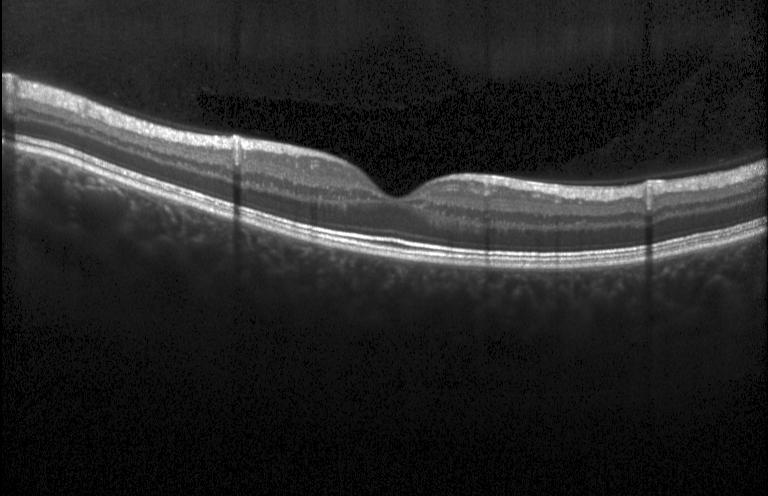
Spectral-domain optical coherence tomography, macular scan, Heidelberg Spectralis OCT system, OCT line scan.
No choroidal neovascularization, diabetic macular edema, or drusen.